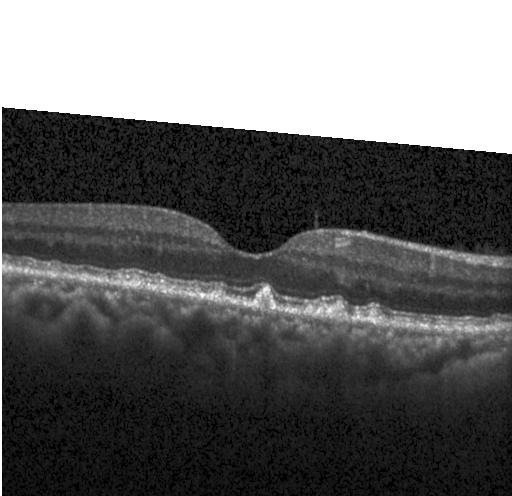 Heidelberg Spectralis; spectral-domain OCT; macular scan; optical coherence tomography B-scan.
Impression: multiple drusen.